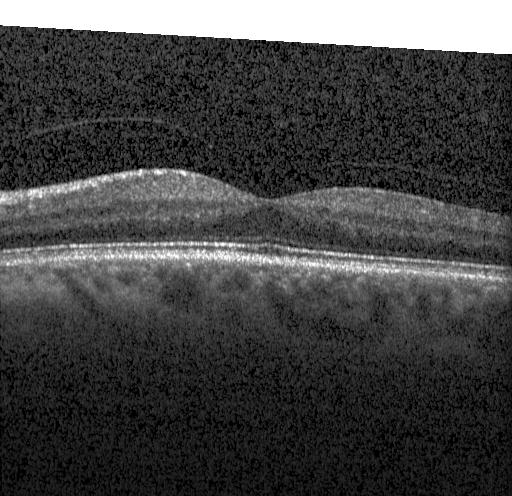

Macular OCT: neither choroidal neovascularization, diabetic macular edema, nor drusen.